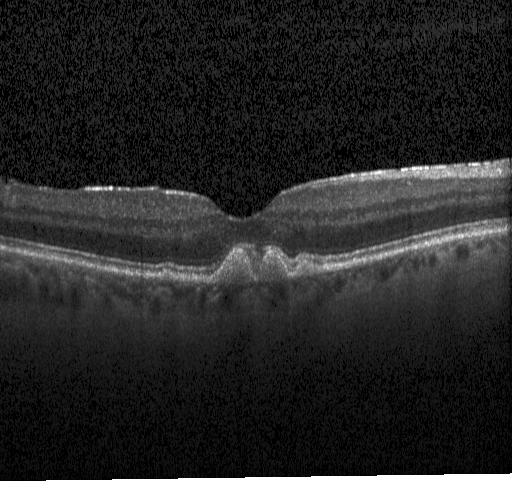
Retinal OCT cross-section · spectral-domain optical coherence tomography · horizontal scan through the fovea — Impression: drusen.